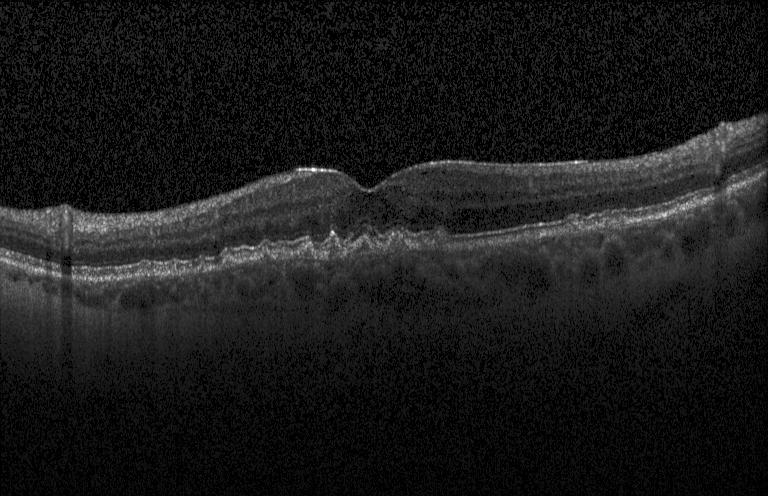 SD-OCT; optical coherence tomography B-scan; Heidelberg Spectralis; horizontal scan through the fovea.
Finding: drusen.